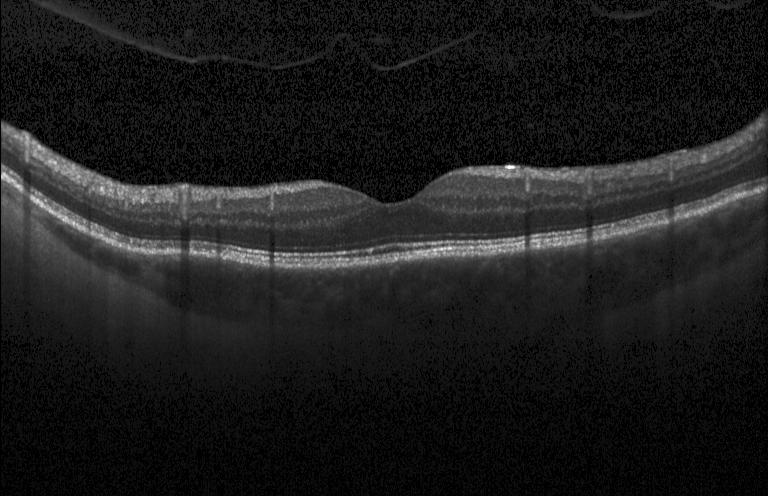 OCT scan showing no choroidal neovascularization, diabetic macular edema, or drusen.